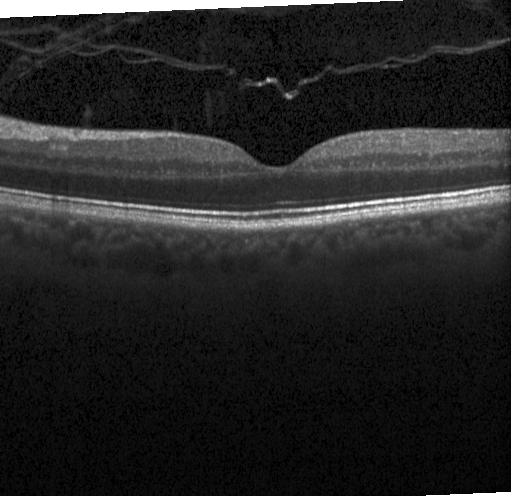 Through the macula. Instrument: Heidelberg Spectralis. Retinal OCT cross-section
Assessment: no evidence of CNV, DME, or drusen.